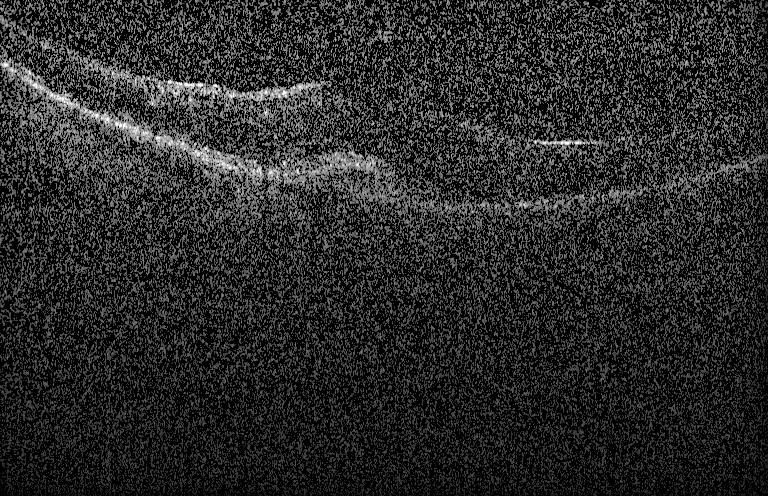
OCT B-scan. Impression: a choroidal neovascular membrane.